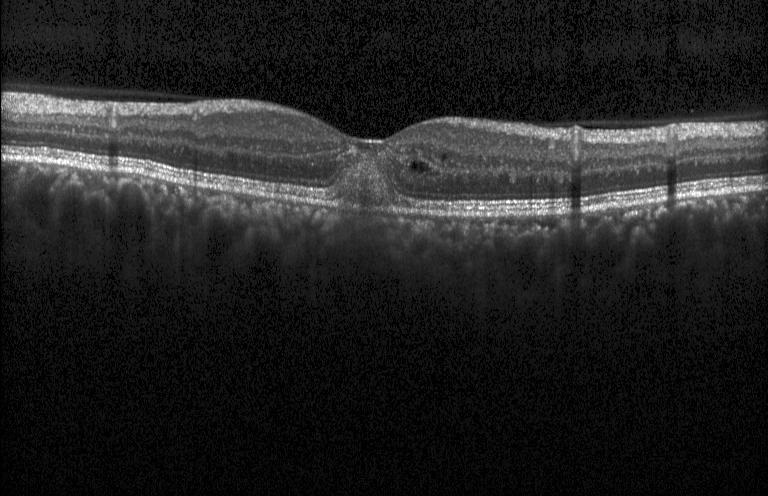
Heidelberg Spectralis, horizontal scan through the fovea, spectral-domain optical coherence tomography, retinal OCT cross-section.
Finding: CNV.